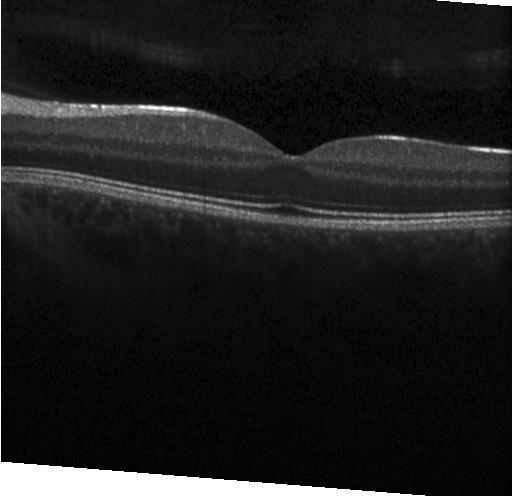
Spectral-domain OCT, macular scan, retinal OCT B-scan.
Diagnosis: neither choroidal neovascularization, diabetic macular edema, nor drusen.